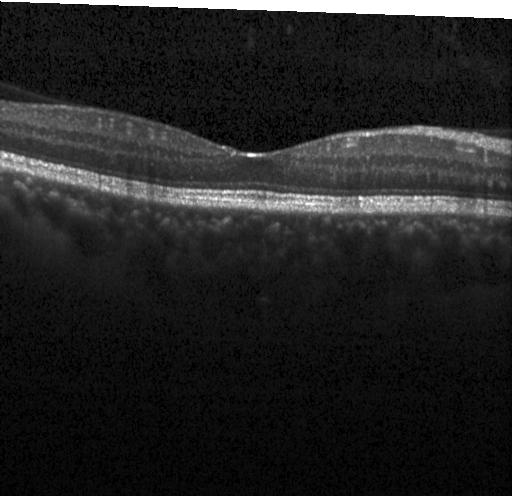
Finding: no CNV, DME, or drusen.